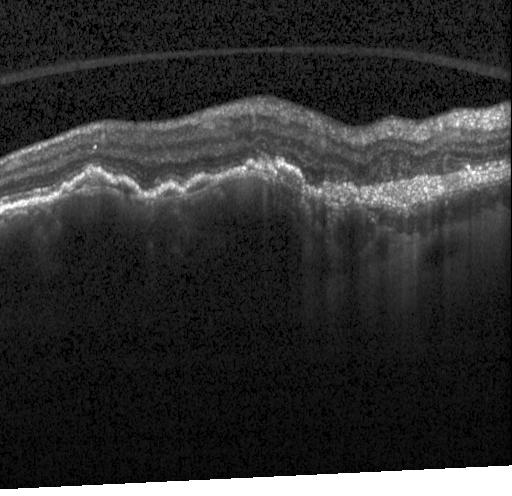
Diagnosis: a choroidal neovascular membrane.